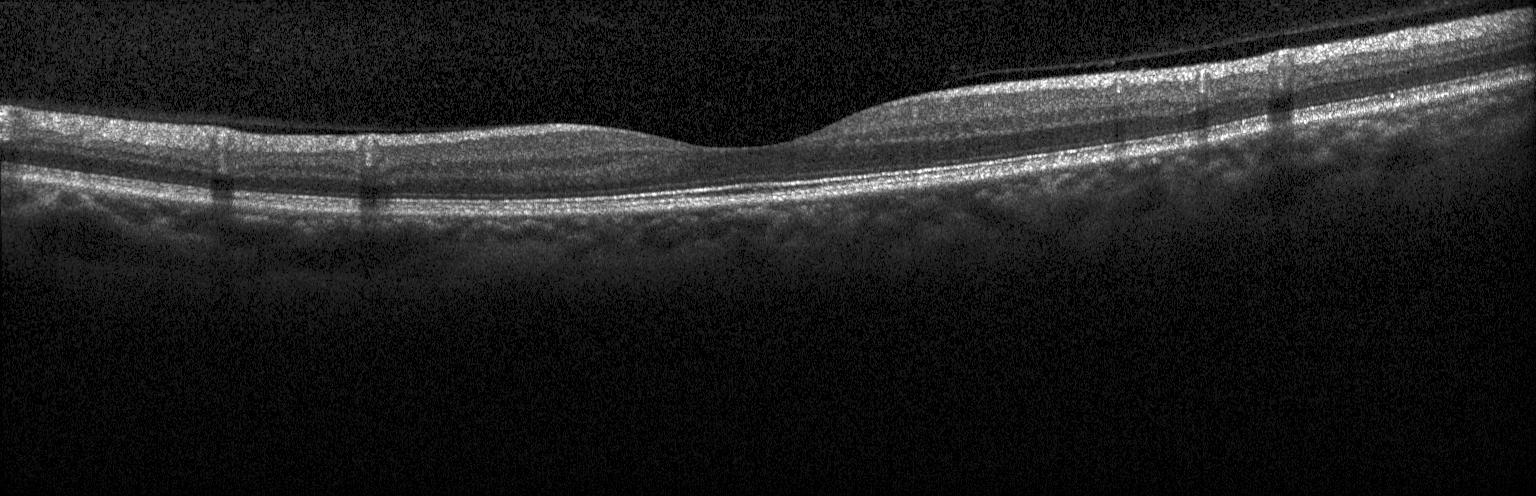 Retinal OCT cross-section
Diagnosis: no evidence of CNV, DME, or drusen.